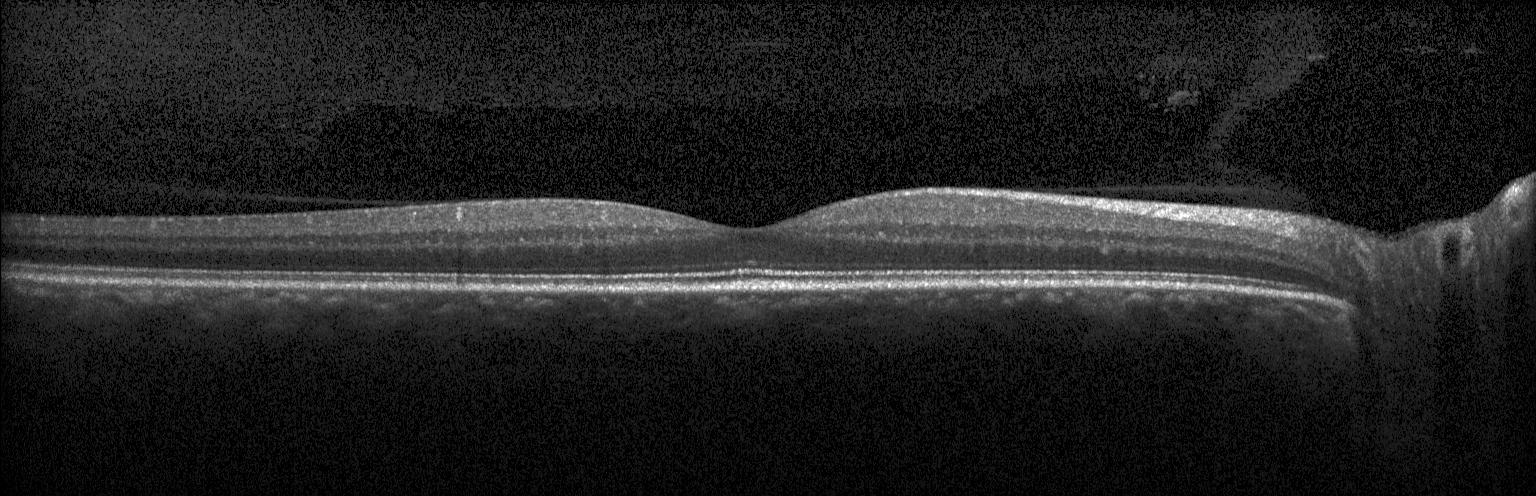 Optical coherence tomography B-scan. Impression: no evidence of CNV, DME, or drusen.